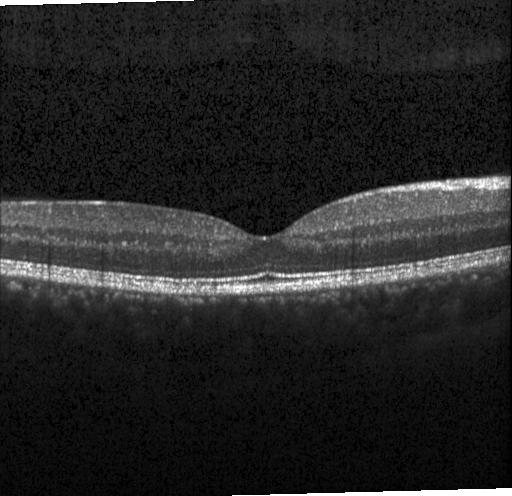 OCT B-scan showing no evidence of choroidal neovascularization, diabetic macular edema, or drusen.